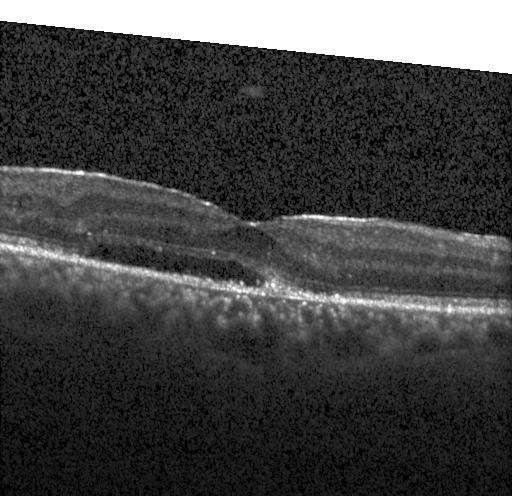
Spectral-domain OCT B-scan: choroidal neovascularization (CNV).